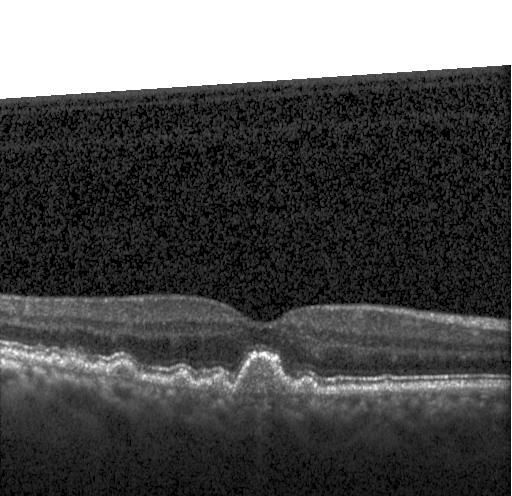

OCT line scan — Macular OCT: multiple drusen.